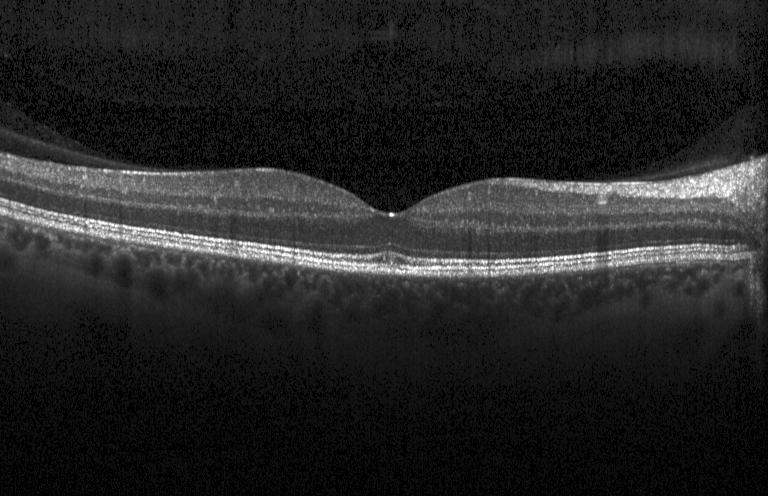

Finding: no choroidal neovascularization, no diabetic macular edema, and no drusen.